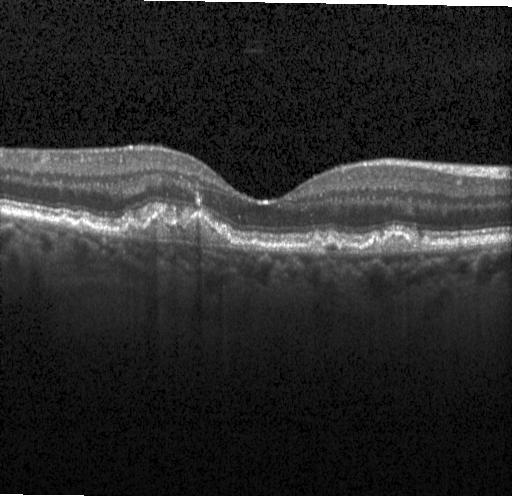
Spectral-domain OCT · retinal OCT cross-section
Macular OCT: choroidal neovascularization.